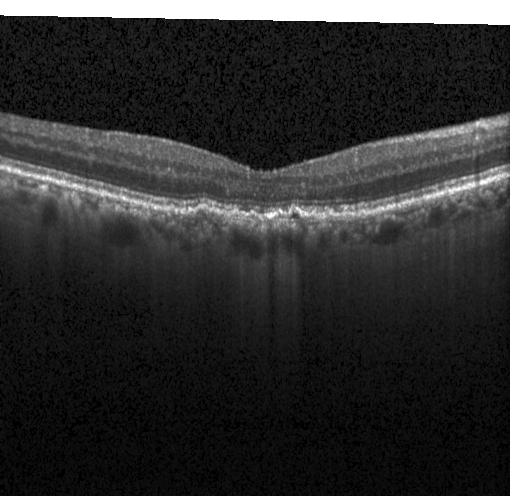

The scan shows sub-RPE drusenoid deposits.